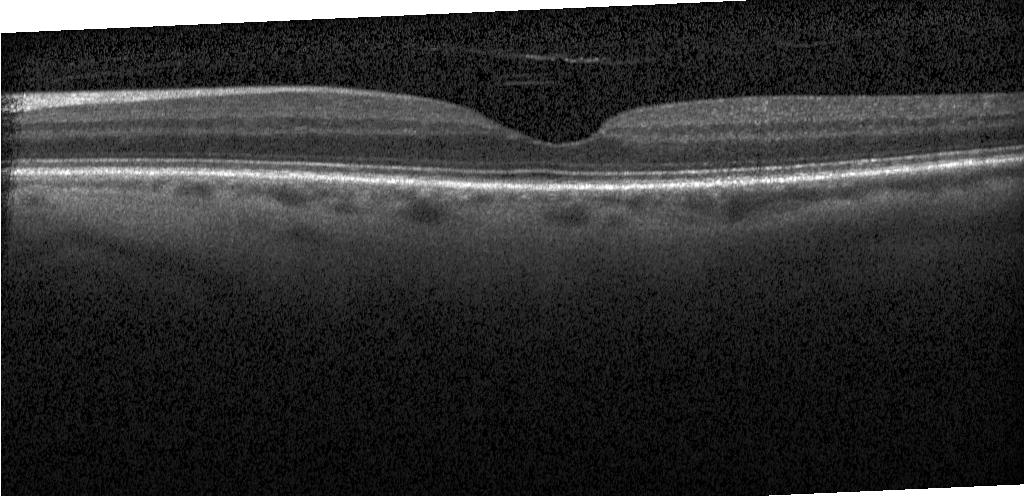
Optical coherence tomography scan. Instrument: Heidelberg Spectralis. Macular scan. Spectral-domain optical coherence tomography. Macular OCT: no CNV, DME, or drusen.